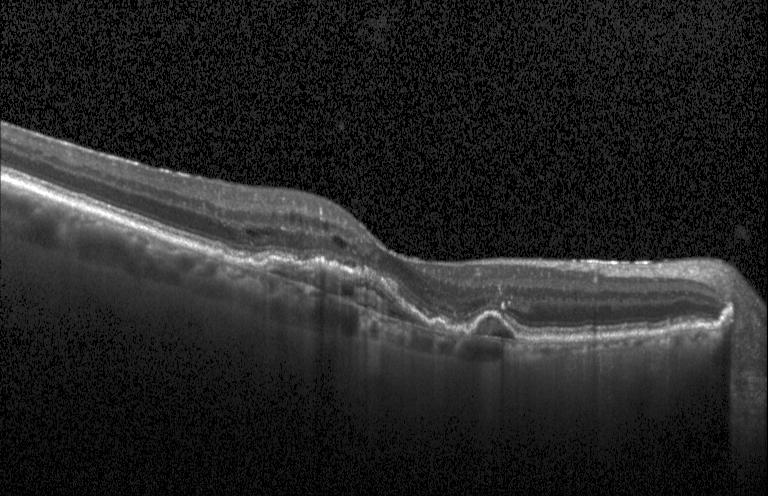 Retinal OCT B-scan
Diagnosis: a choroidal neovascular membrane.